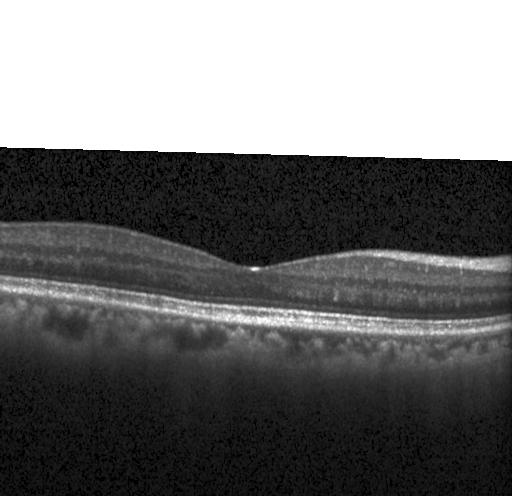 Centered on the fovea, OCT B-scan, spectral-domain optical coherence tomography, Heidelberg Spectralis
This B-scan demonstrates no choroidal neovascularization, diabetic macular edema, or drusen.